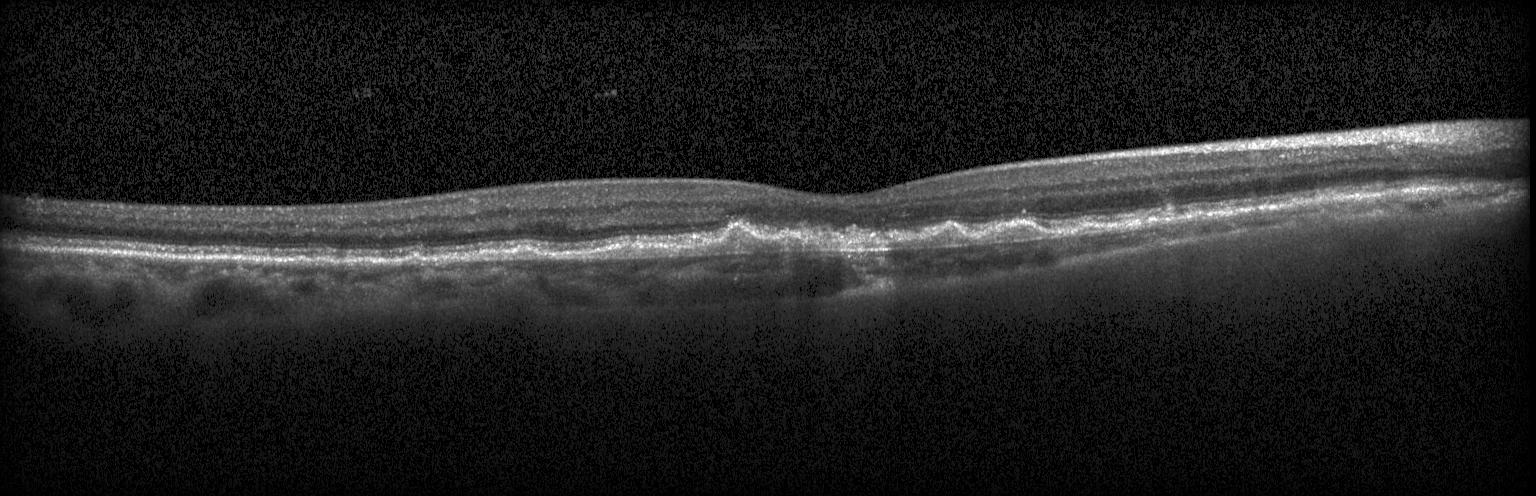
Assessment: choroidal neovascularization (CNV).